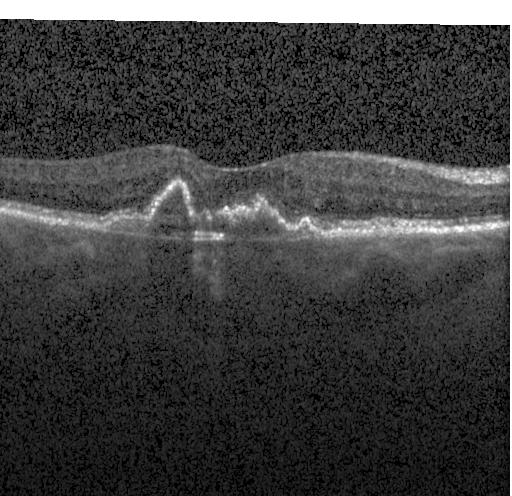

SD-OCT; optical coherence tomography scan; Heidelberg Spectralis OCT system; centered on the fovea
Assessment: a choroidal neovascular membrane.